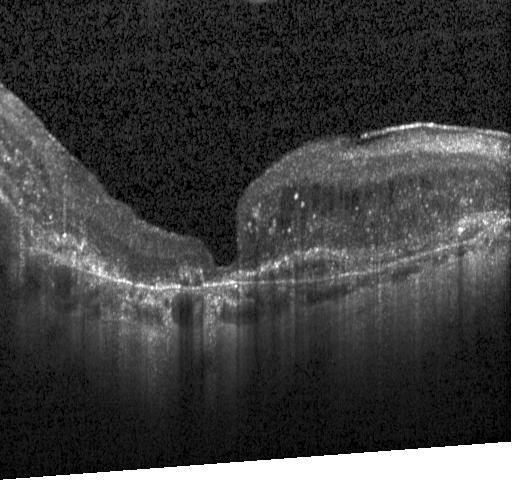
Spectral-domain OCT B-scan: choroidal neovascularization (CNV).